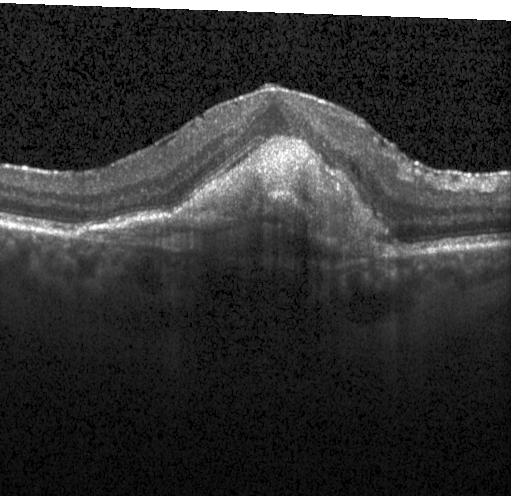 Impression: a choroidal neovascular membrane.